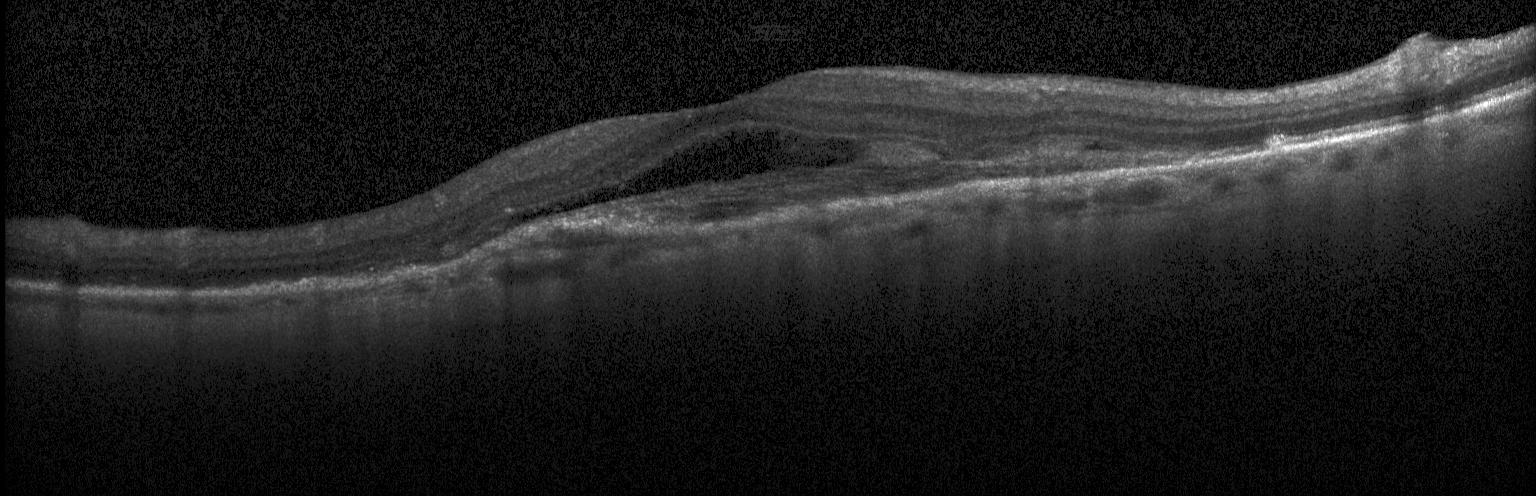 OCT B-scan, Heidelberg Spectralis OCT system, spectral-domain OCT.
Dx: choroidal neovascularization (CNV).